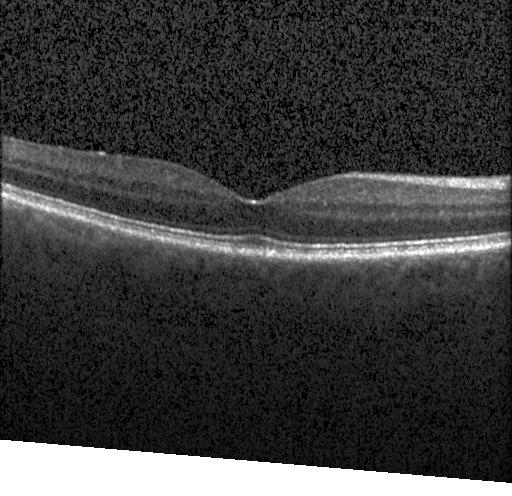

Finding: no CNV, no DME, and no drusen.